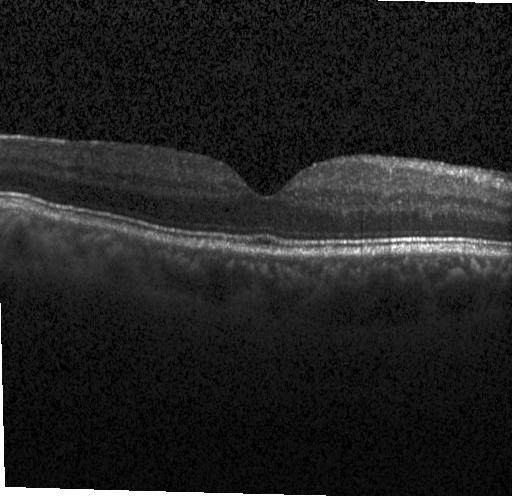
OCT finding: neither CNV, DME, nor drusen.